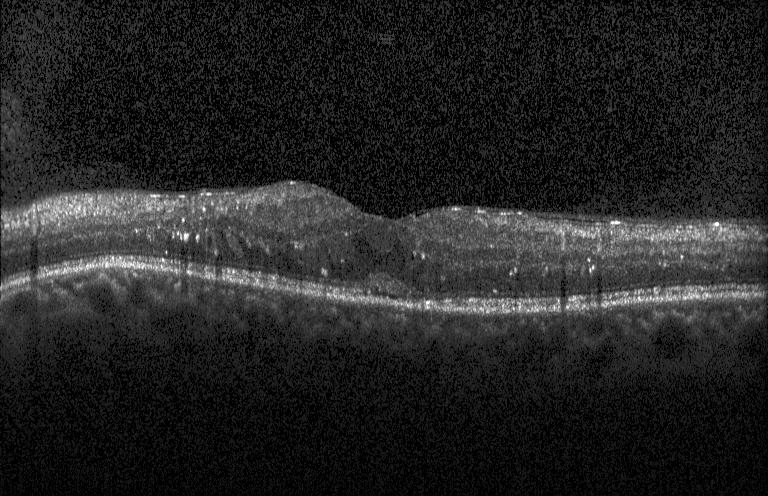 OCT B-scan. Horizontal scan through the fovea — Impression: DME.